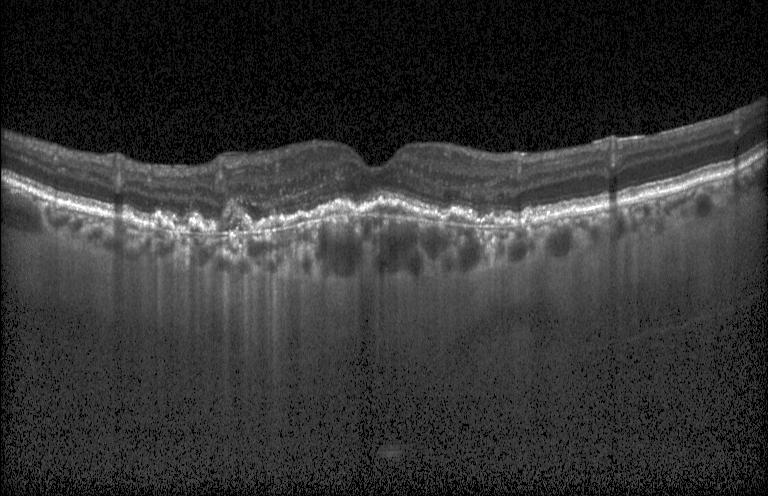
Fovea-centered, instrument: Heidelberg Spectralis, SD-OCT, OCT line scan.
Dx: a choroidal neovascular membrane.